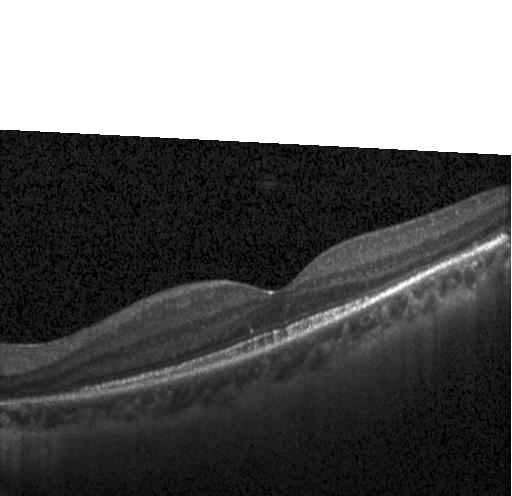 Diagnosis: neither choroidal neovascularization, diabetic macular edema, nor drusen.